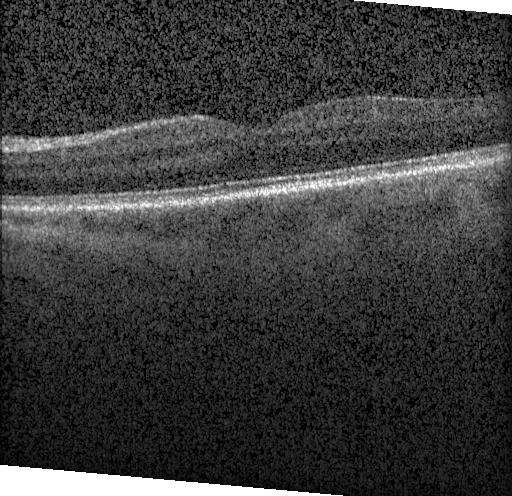

The scan shows no evidence of CNV, DME, or drusen.